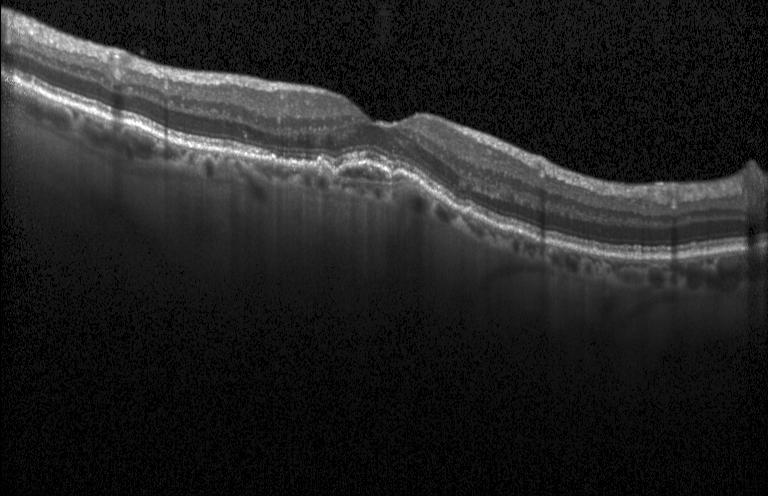 Optical coherence tomography scan.
This B-scan demonstrates a choroidal neovascular membrane.